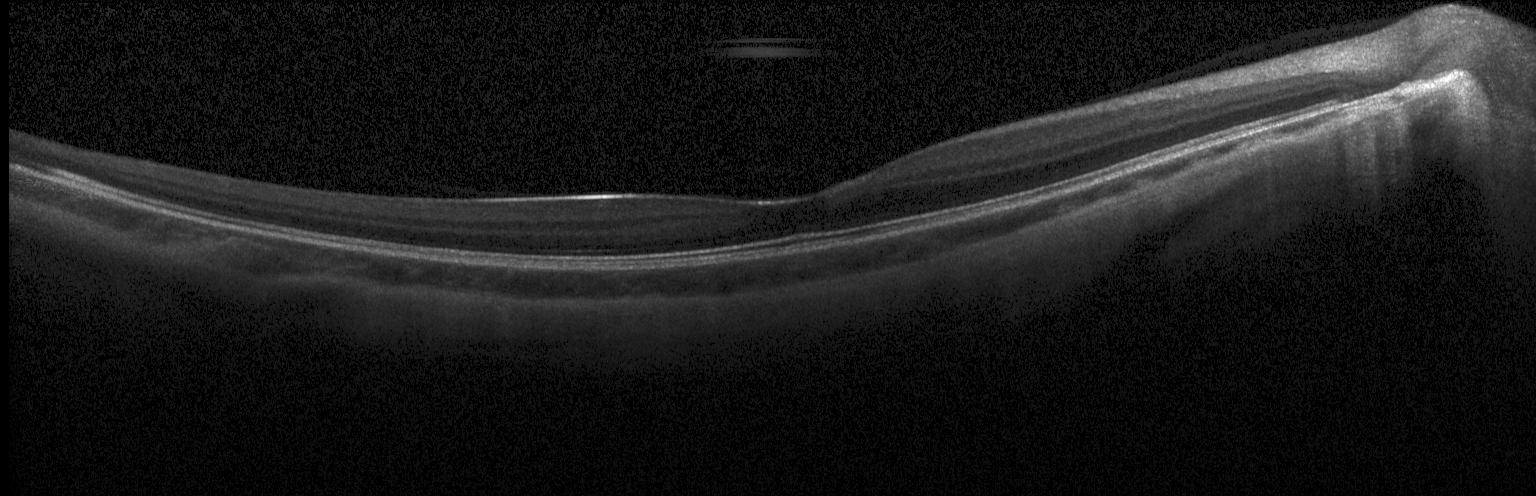
Diagnosis: neither CNV, DME, nor drusen.